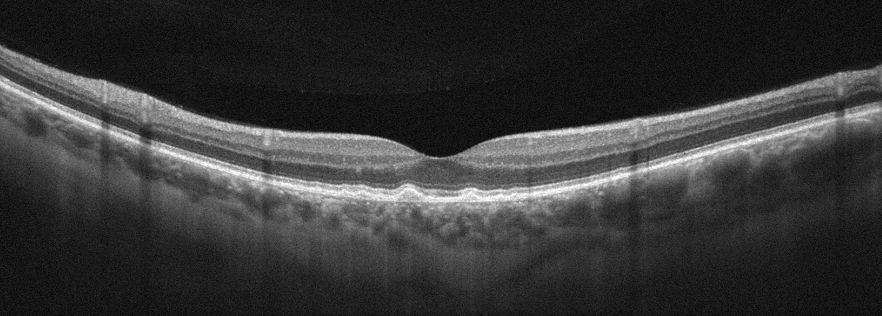 Left eye. Macular scan. Acquired on an Optovue Avanti RTVue XR. Optical coherence tomography scan.
Dx: age-related macular degeneration.